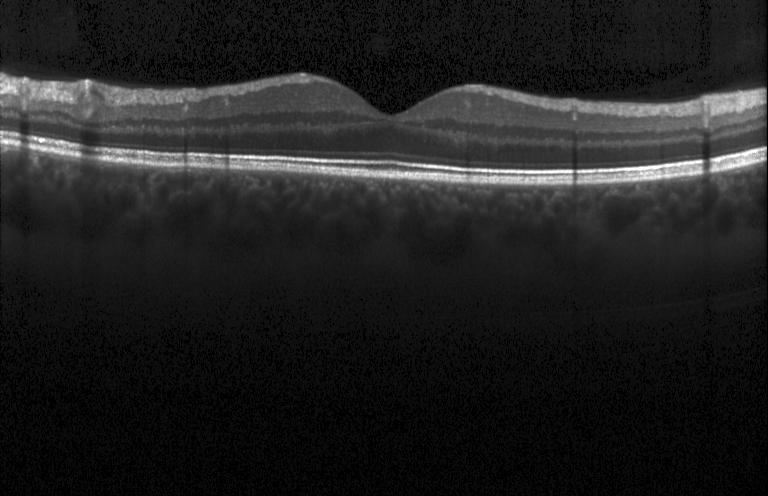
This B-scan demonstrates no choroidal neovascularization, diabetic macular edema, or drusen.